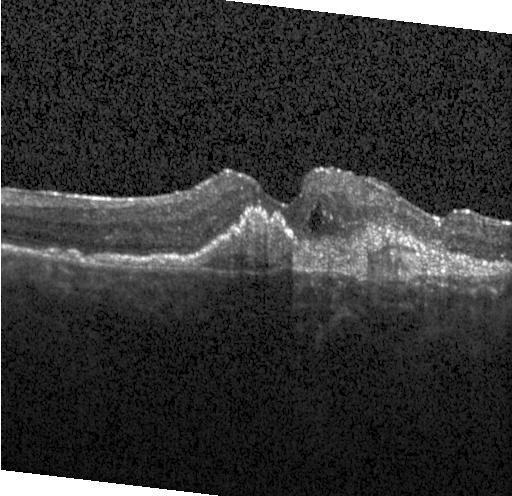

Optical coherence tomography B-scan; Heidelberg Spectralis; fovea-centered.
A choroidal neovascular membrane.